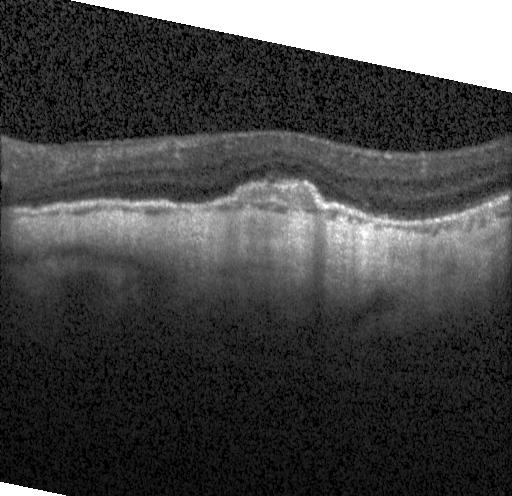

Retinal OCT cross-section showing a choroidal neovascular membrane.